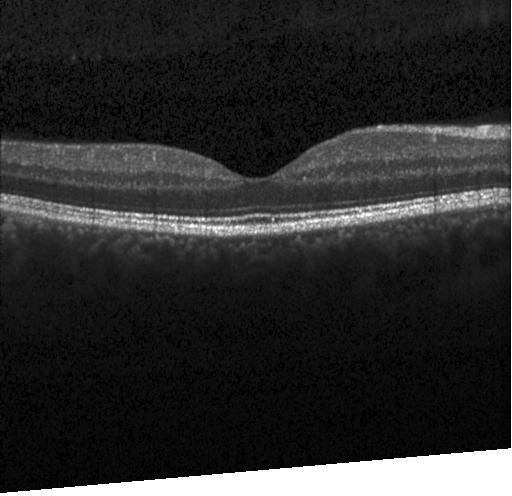
Heidelberg Spectralis OCT system. Spectral-domain OCT. Retinal OCT B-scan
No choroidal neovascularization, diabetic macular edema, or drusen.